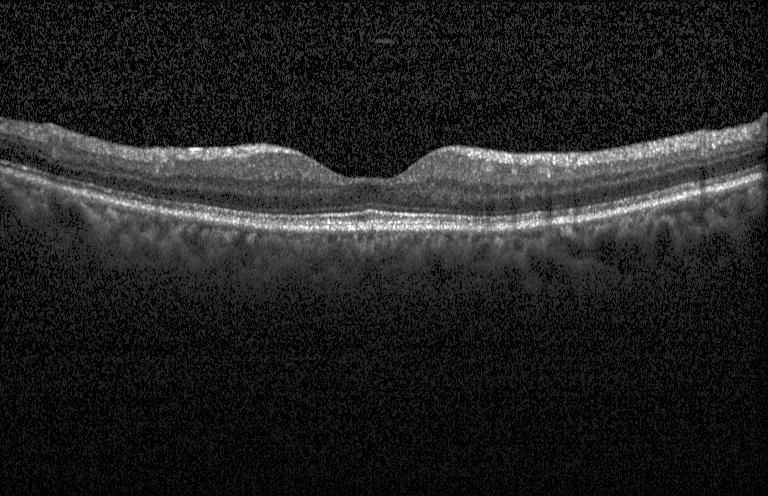 Retinal OCT cross-section. Heidelberg Spectralis OCT system. Spectral-domain OCT.
The scan shows neither choroidal neovascularization, diabetic macular edema, nor drusen.